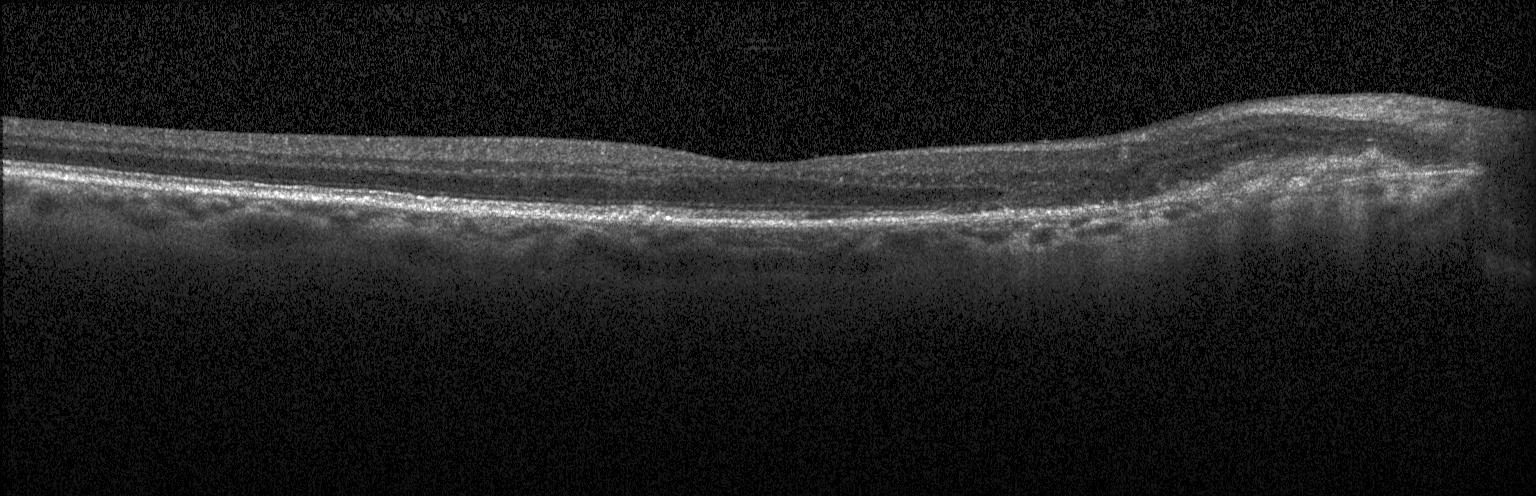

Finding: CNV.